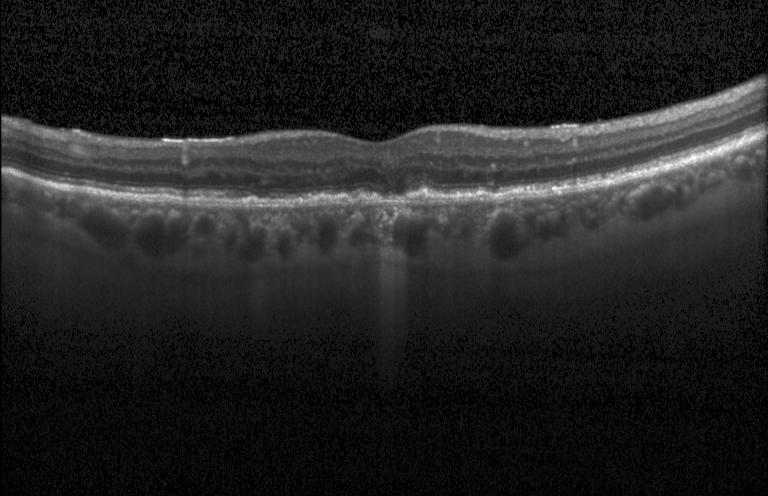 Spectral-domain OCT · OCT line scan
Dx: a choroidal neovascular membrane.